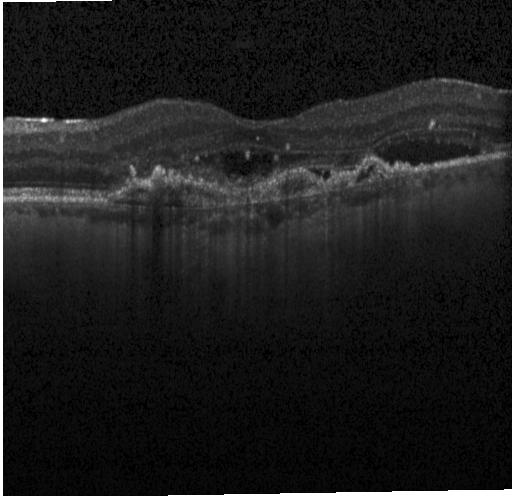 Spectral-domain OCT, OCT B-scan, through the macula.
Assessment: CNV.